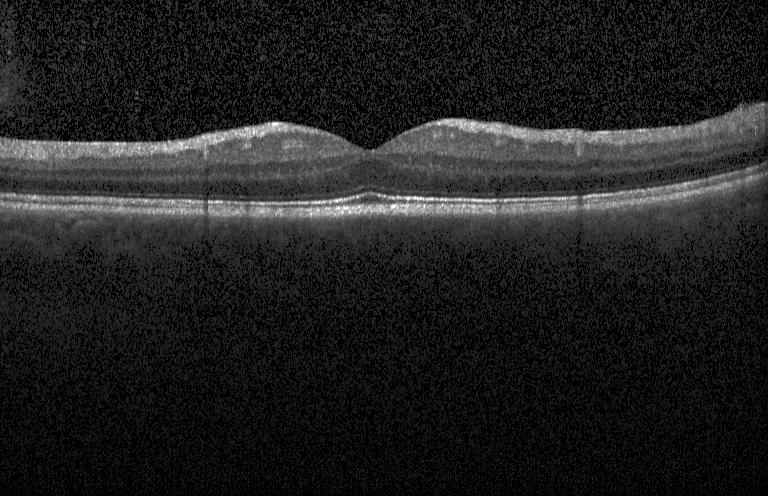 Finding: neither CNV, DME, nor drusen.